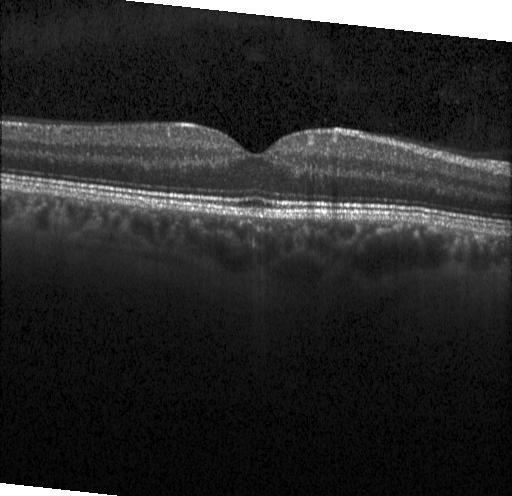
Spectral-domain OCT B-scan: neither choroidal neovascularization, diabetic macular edema, nor drusen.